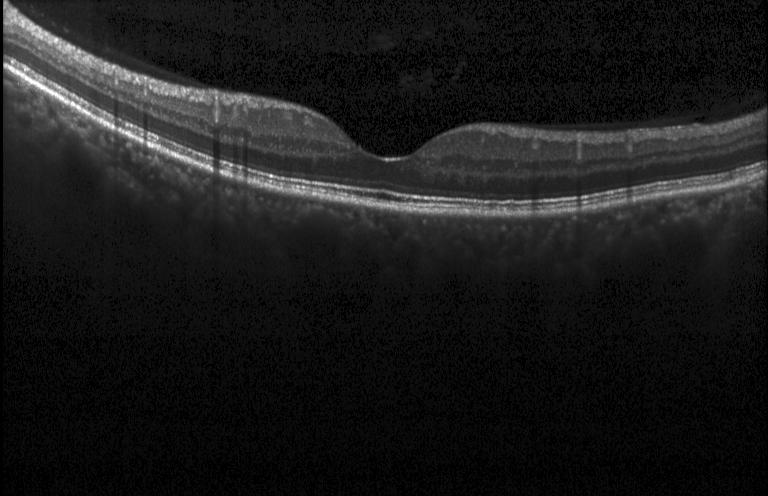 Finding: no choroidal neovascularization, diabetic macular edema, or drusen.